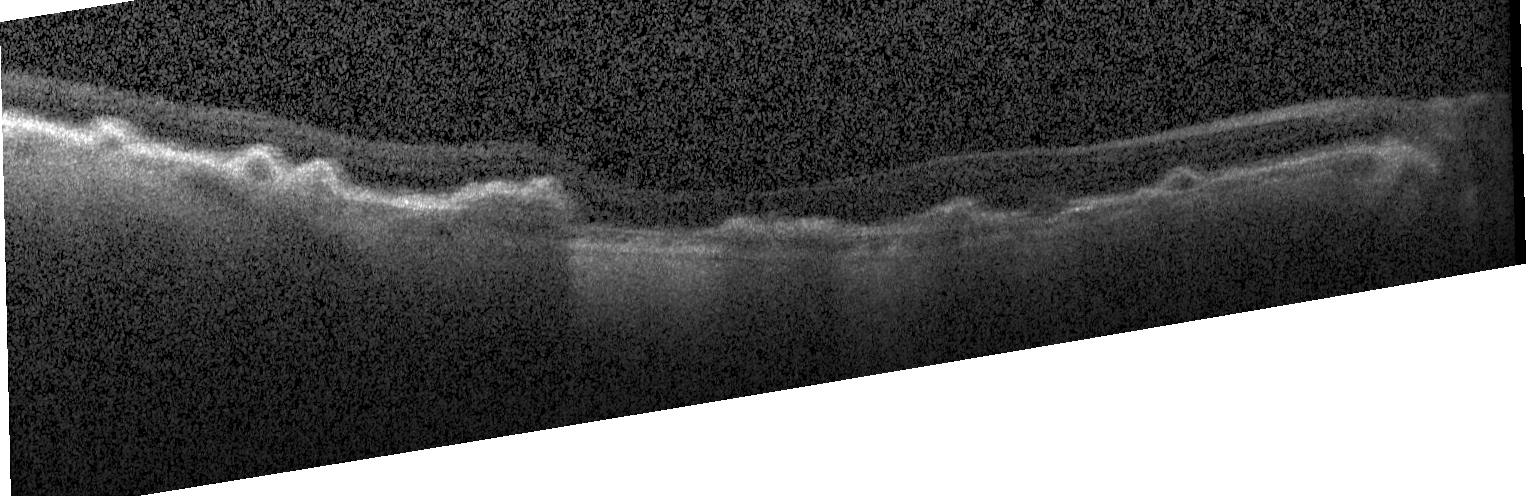
Finding: choroidal neovascularization.